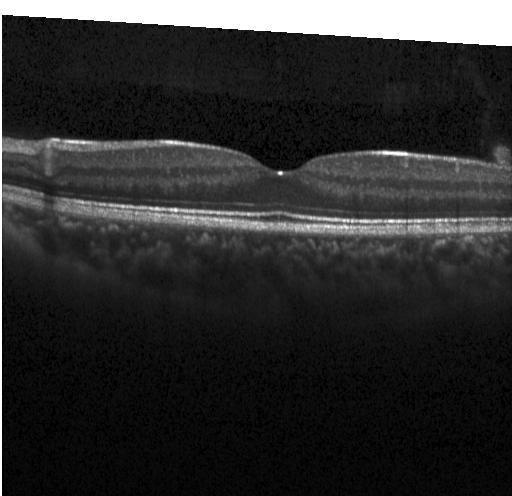
Optical coherence tomography scan · macular scan
Dx: no choroidal neovascularization, diabetic macular edema, or drusen.